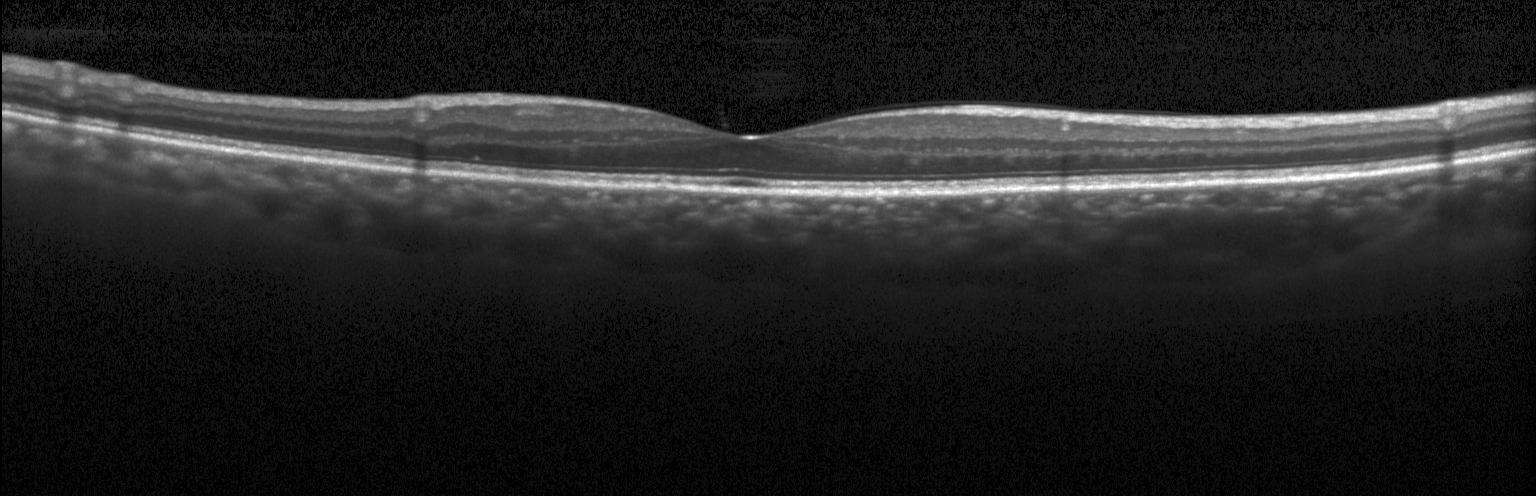
Heidelberg Spectralis OCT system, OCT B-scan. Finding: no evidence of choroidal neovascularization, diabetic macular edema, or drusen.